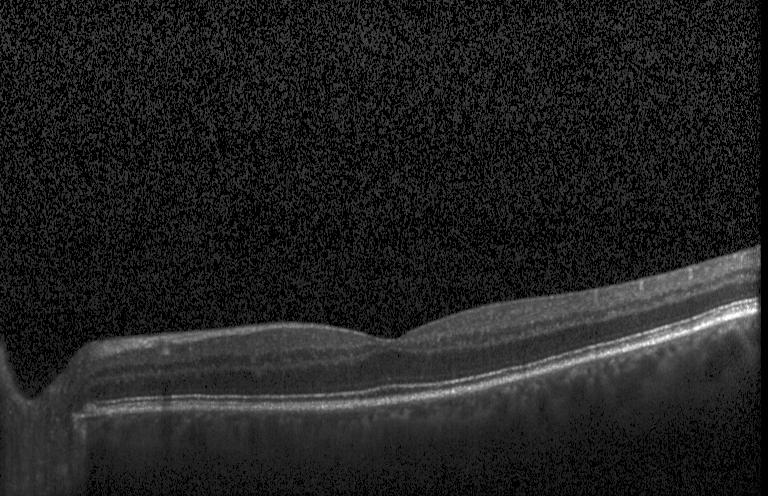 Dx: neither choroidal neovascularization, diabetic macular edema, nor drusen.